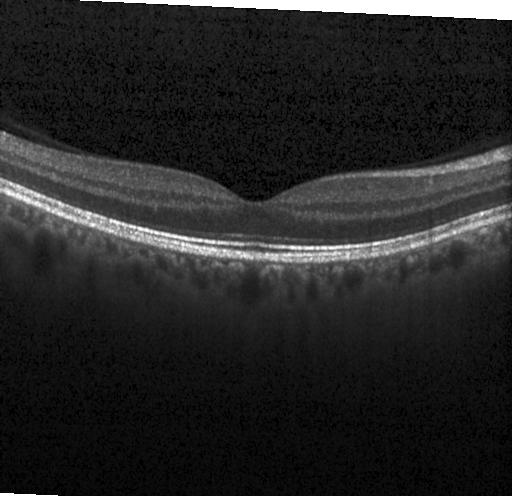 Finding: no choroidal neovascularization, no diabetic macular edema, and no drusen.